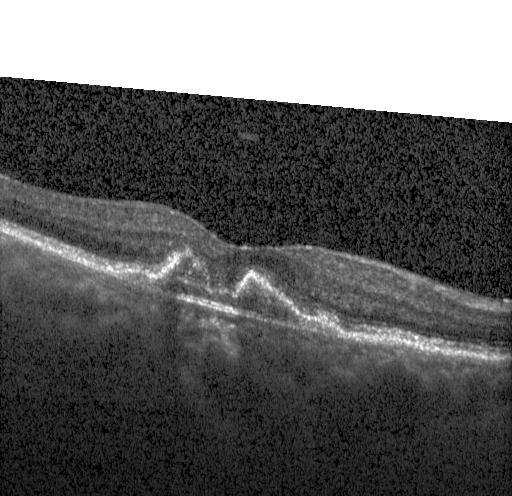

Horizontal scan through the fovea; OCT line scan.
Diagnosis: a choroidal neovascular membrane.